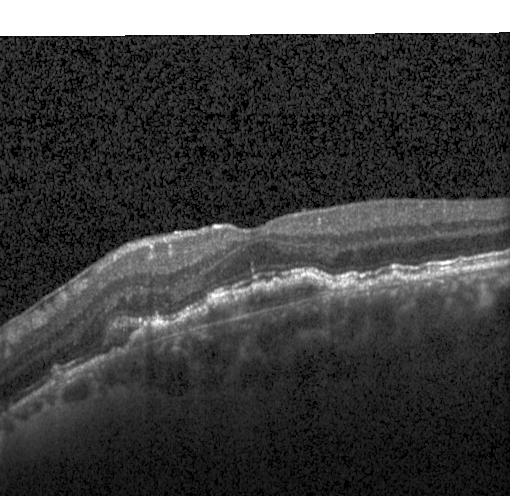
Finding: choroidal neovascularization.